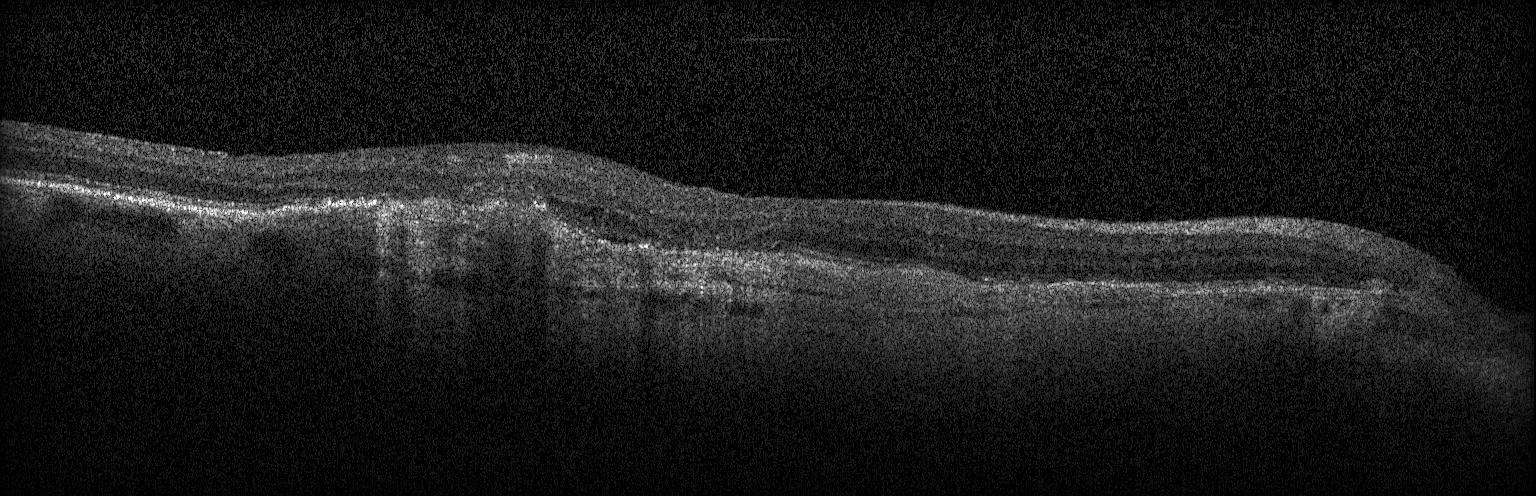 OCT B-scan — Diagnosis: choroidal neovascularization (CNV).